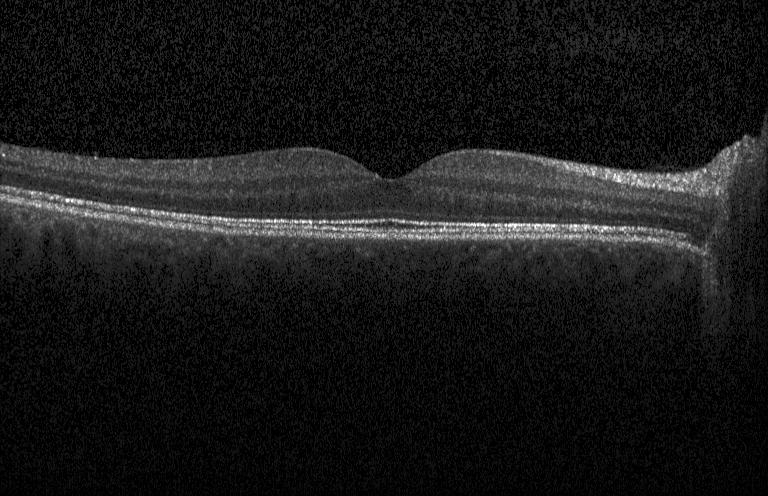

No choroidal neovascularization, no diabetic macular edema, and no drusen.